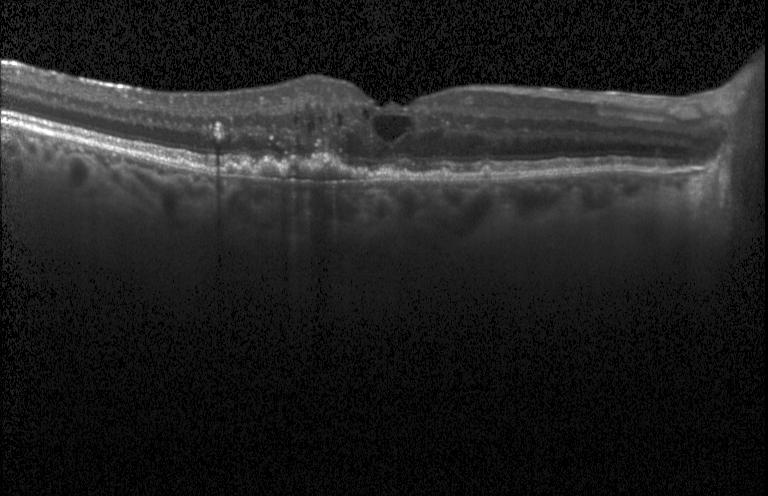

Heidelberg Spectralis OCT system; fovea-centered; spectral-domain OCT; OCT B-scan. Finding: CNV.